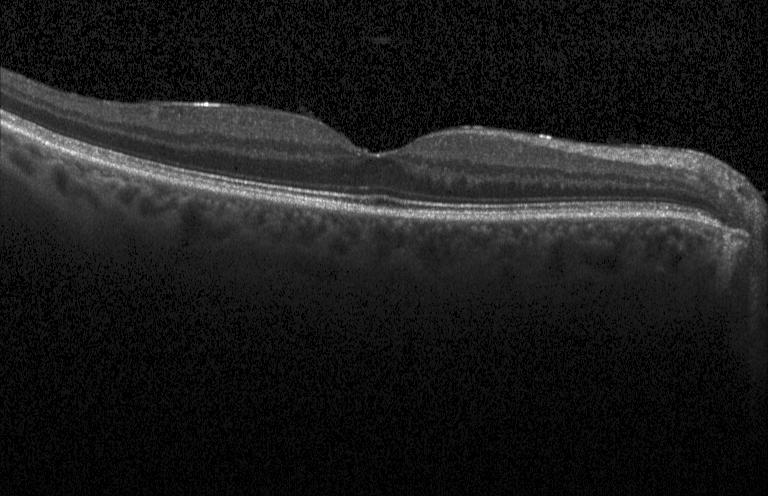

Retinal OCT B-scan, through the macula. The scan shows no evidence of choroidal neovascularization, diabetic macular edema, or drusen.